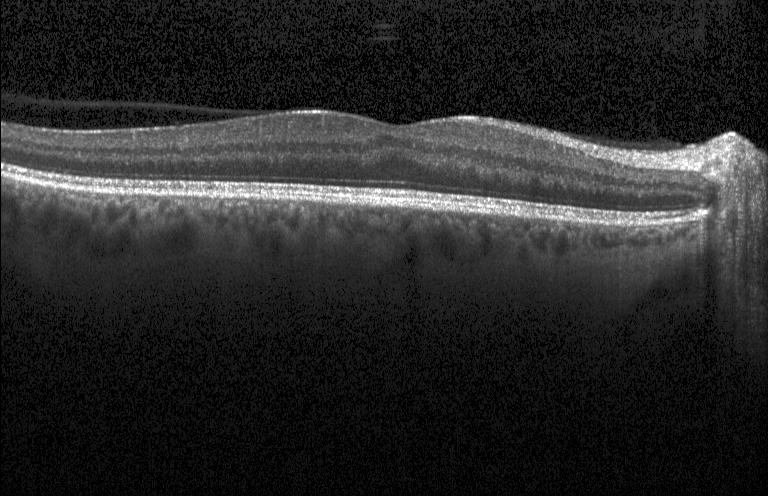

Through the macula; SD-OCT; instrument: Heidelberg Spectralis; optical coherence tomography B-scan
Diagnosis: no choroidal neovascularization, diabetic macular edema, or drusen.